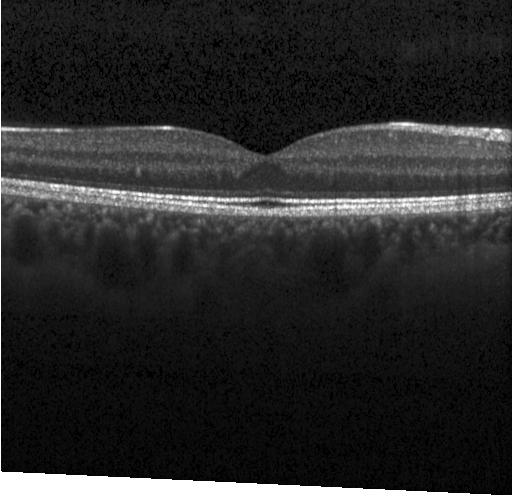
This B-scan demonstrates no evidence of choroidal neovascularization, diabetic macular edema, or drusen.